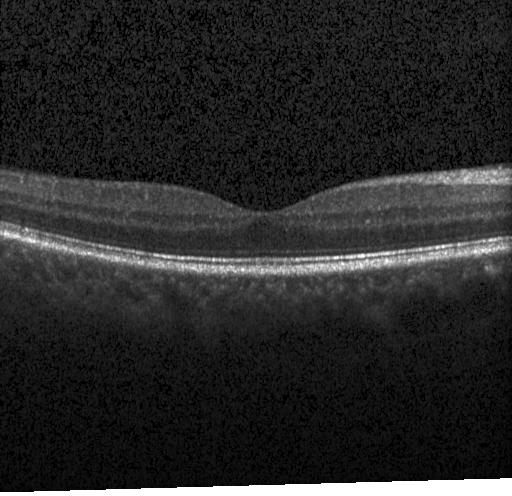
OCT finding: no choroidal neovascularization, diabetic macular edema, or drusen.